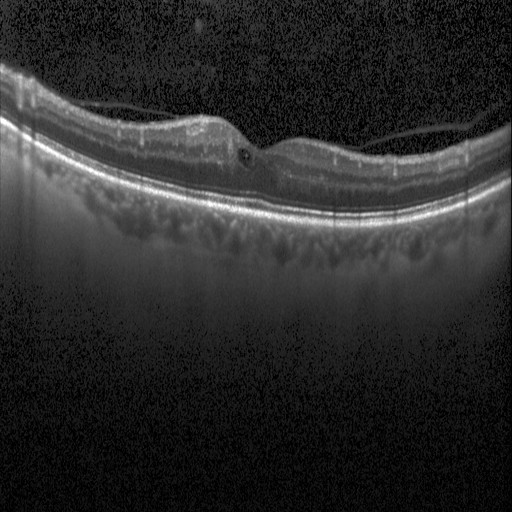 OCT B-scan
Impression: DME.